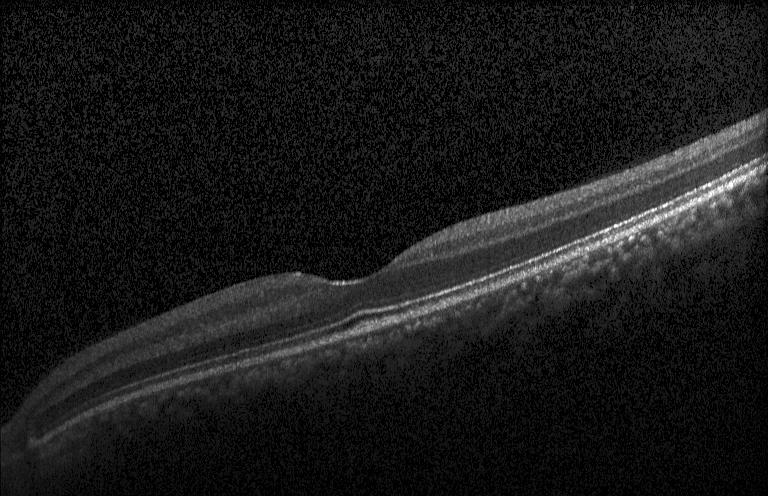 Dx: neither choroidal neovascularization, diabetic macular edema, nor drusen.